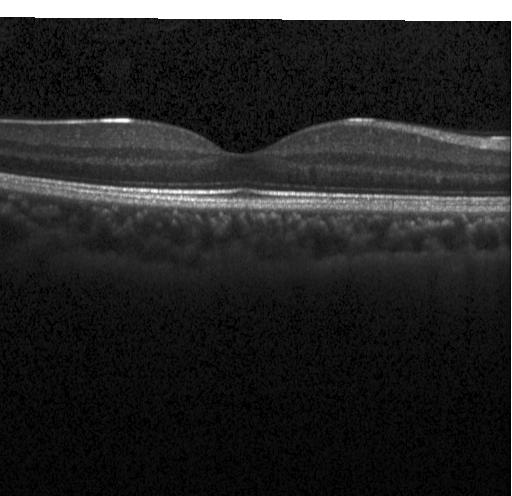

OCT B-scan, acquired on a Heidelberg Spectralis, centered on the fovea. Impression: no evidence of choroidal neovascularization, diabetic macular edema, or drusen.